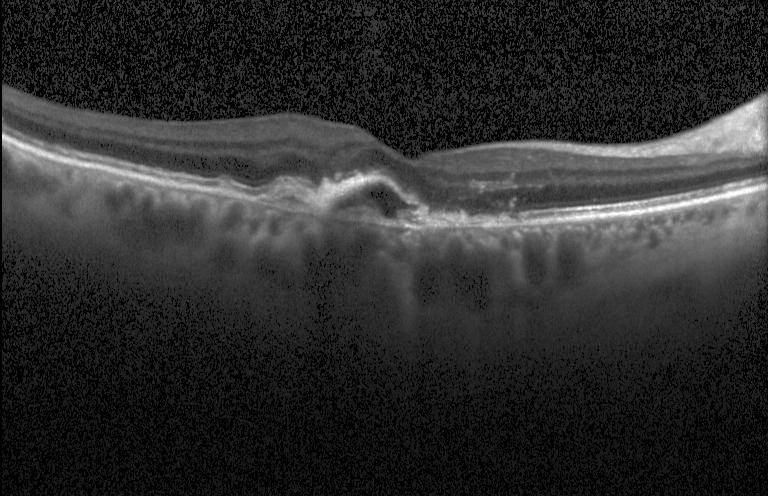 Heidelberg Spectralis OCT system · optical coherence tomography B-scan.
This B-scan demonstrates choroidal neovascularization (CNV).